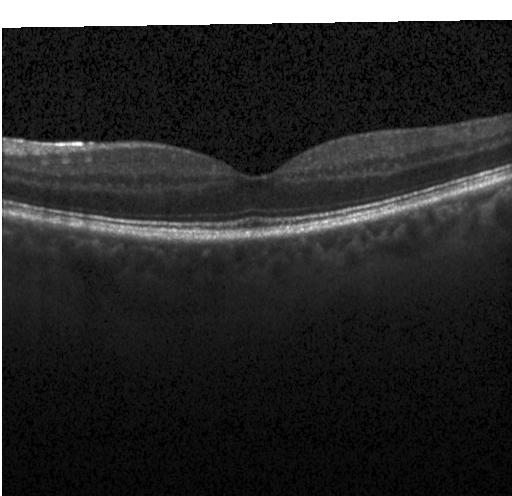

OCT line scan. Fovea-centered. Acquired on a Heidelberg Spectralis. Diagnosis: no evidence of choroidal neovascularization, diabetic macular edema, or drusen.